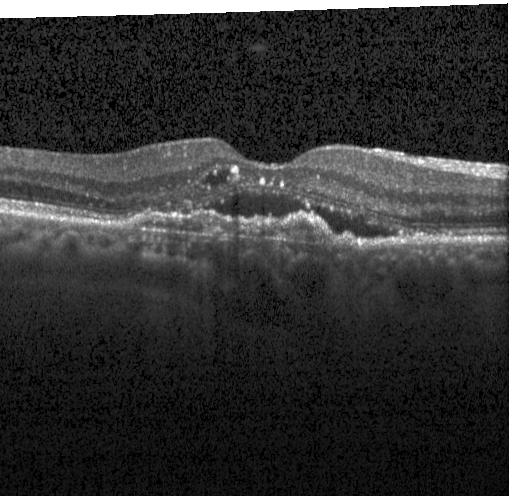 Centered on the fovea. OCT B-scan. Acquired on a Heidelberg Spectralis
Diagnosis: a choroidal neovascular membrane.